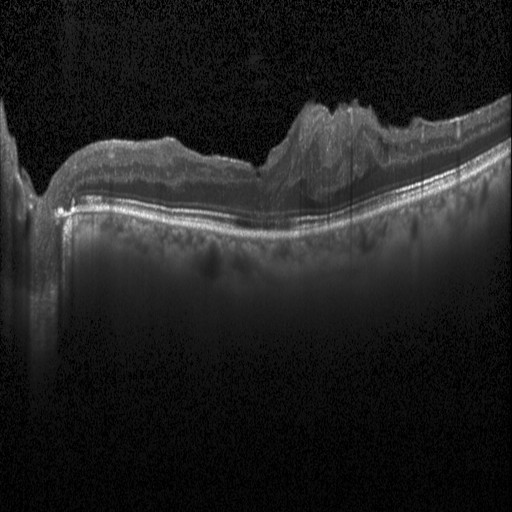 Retinal OCT cross-section. Spectral-domain OCT. Macular scan. Finding: diabetic macular edema (DME).